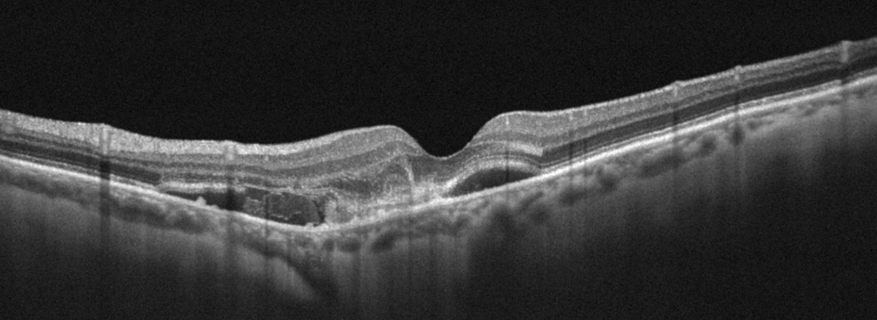 OCT B-scan
Dx: age-related macular degeneration (AMD).